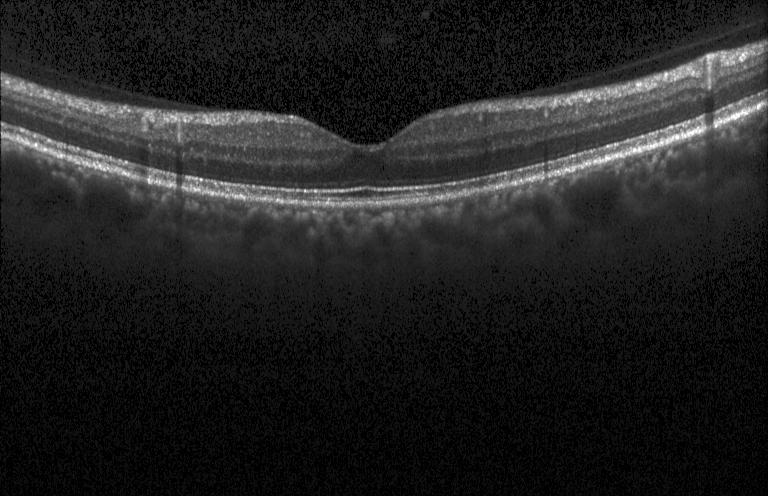

Macular OCT demonstrating no choroidal neovascularization, diabetic macular edema, or drusen.